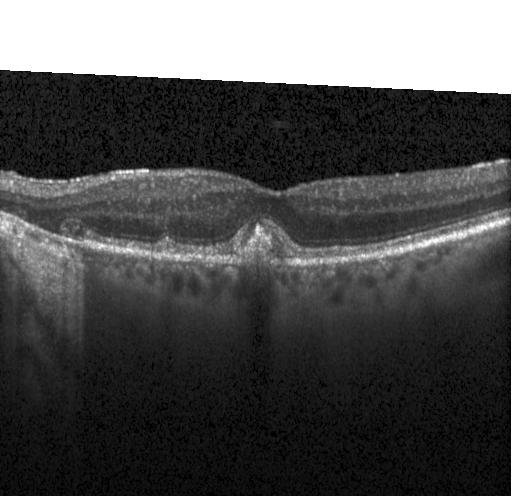

Macular scan; optical coherence tomography B-scan.
This B-scan demonstrates choroidal neovascularization (CNV).